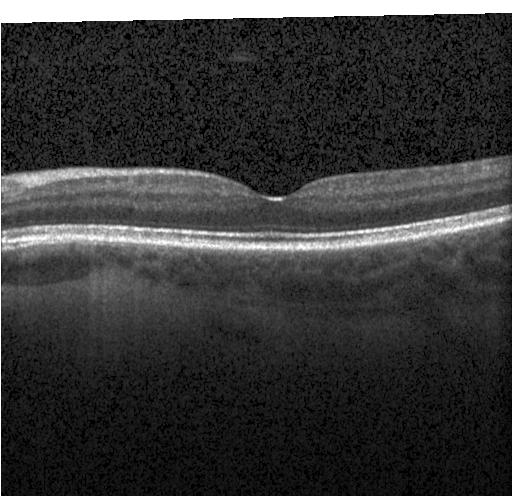 The scan shows no choroidal neovascularization, diabetic macular edema, or drusen.